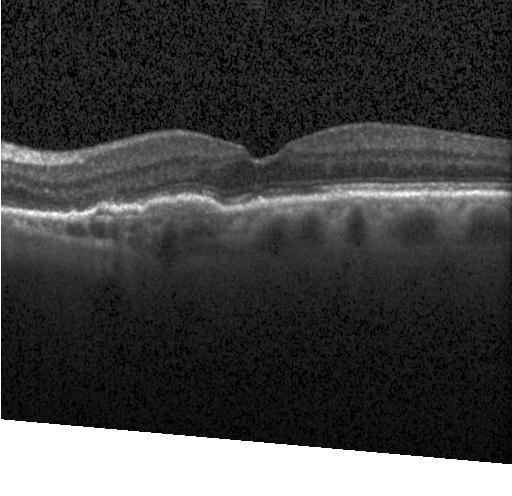 Retinal OCT cross-section showing a choroidal neovascular membrane.